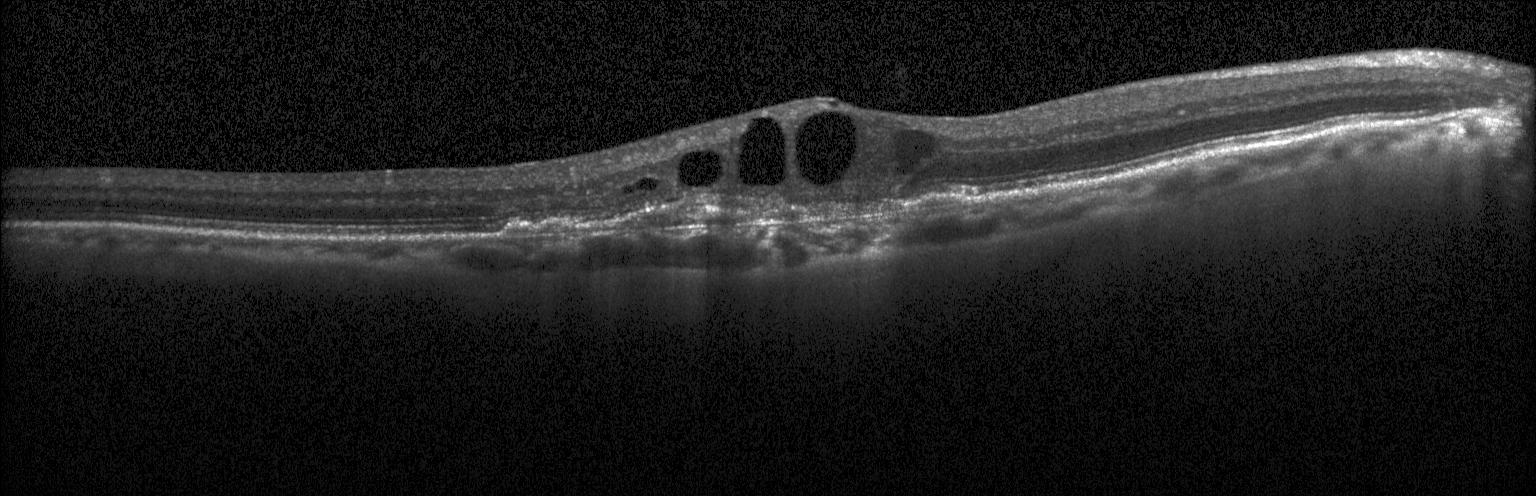 Diagnosis: choroidal neovascularization.